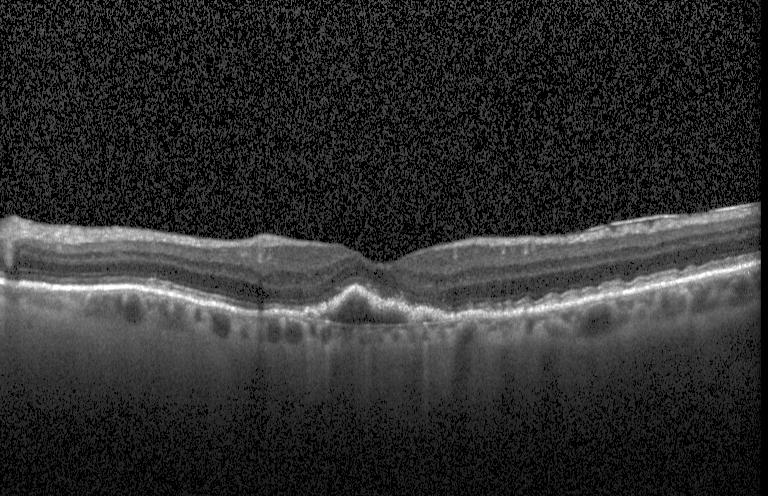

Choroidal neovascularization.